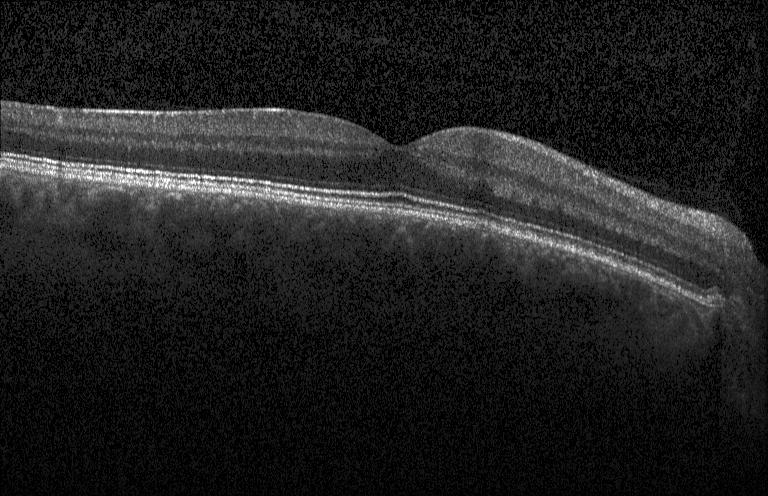 Impression: no choroidal neovascularization, diabetic macular edema, or drusen.